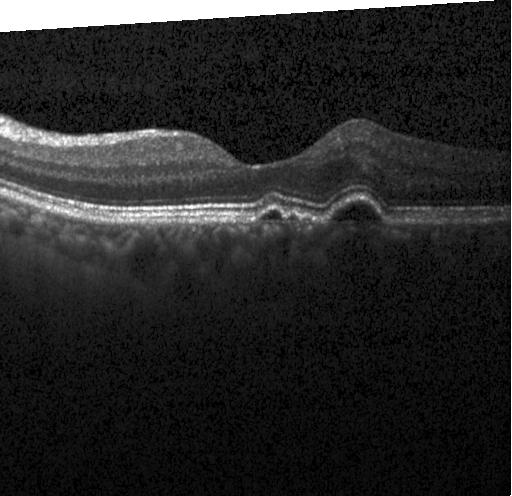 Diagnosis: CNV.